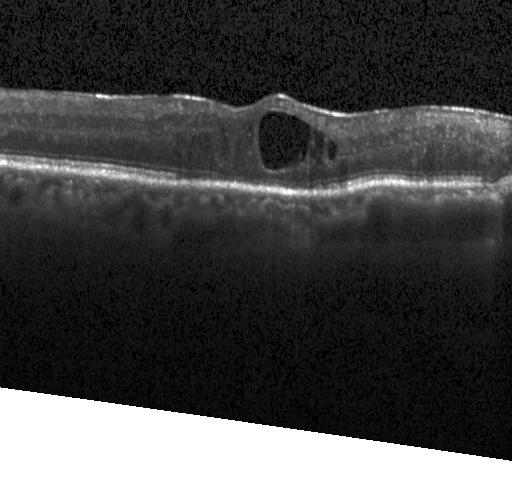

Optical coherence tomography scan
This B-scan demonstrates diabetic macular edema (DME).